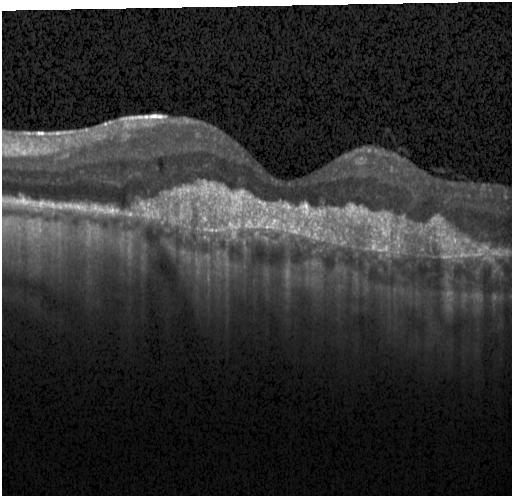 Impression: a choroidal neovascular membrane.